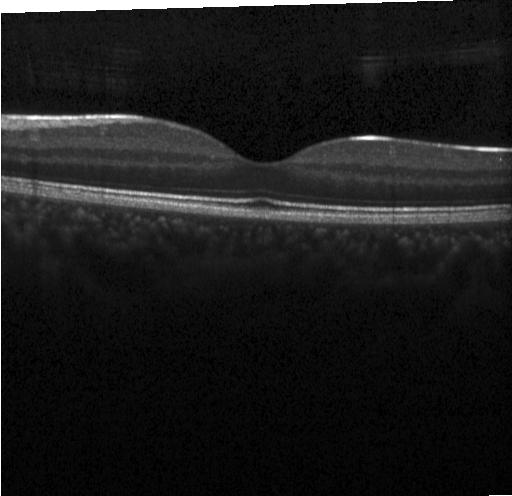
Through the macula, SD-OCT, retinal OCT B-scan, instrument: Heidelberg Spectralis. This B-scan demonstrates no CNV, no DME, and no drusen.